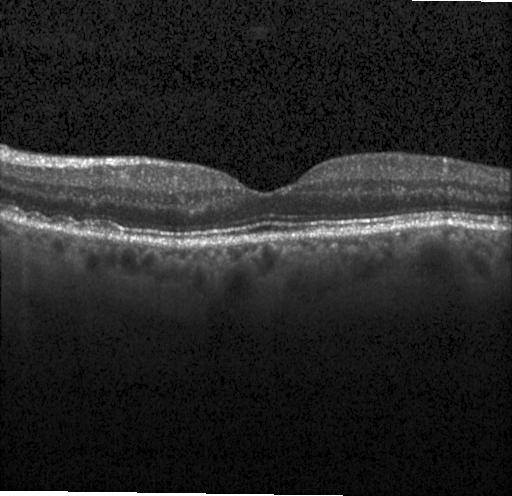

Finding: drusen.